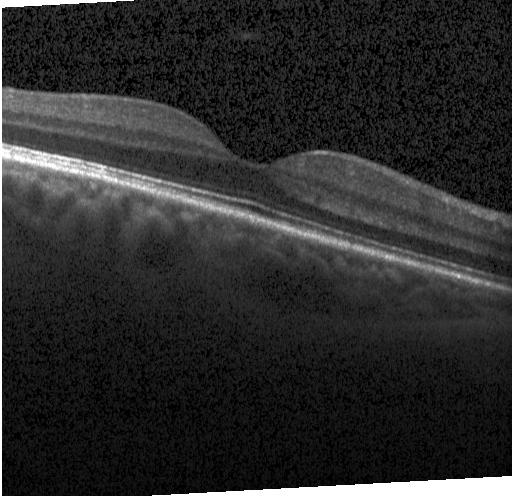 Diagnosis: no choroidal neovascularization, diabetic macular edema, or drusen.